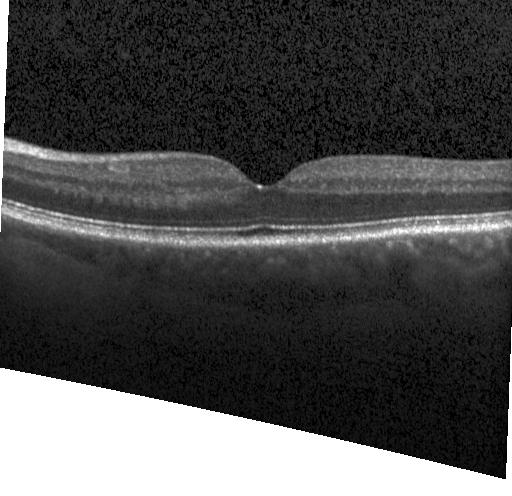

OCT scan showing neither choroidal neovascularization, diabetic macular edema, nor drusen.